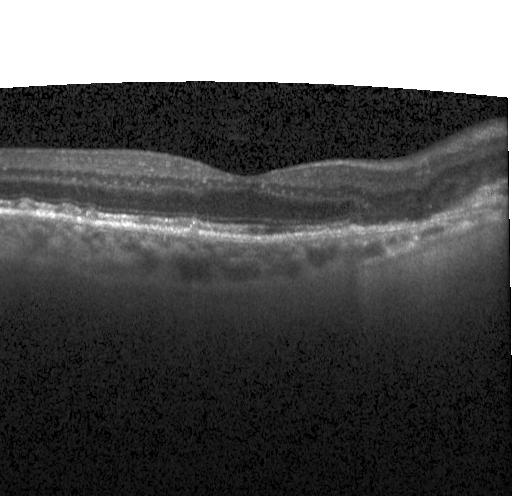

Retinal OCT B-scan; centered on the fovea; Heidelberg Spectralis OCT system; spectral-domain OCT.
The scan shows CNV.